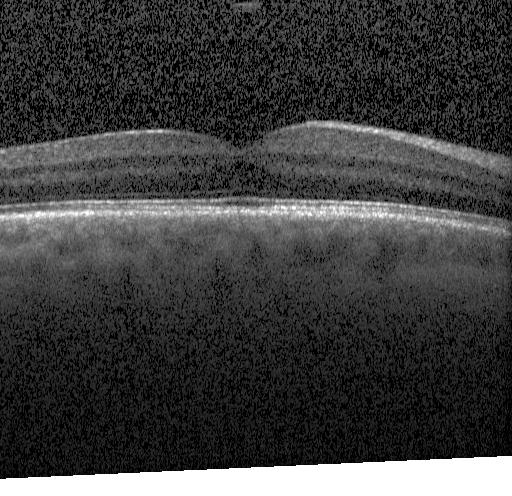

Macular OCT demonstrating no evidence of choroidal neovascularization, diabetic macular edema, or drusen.